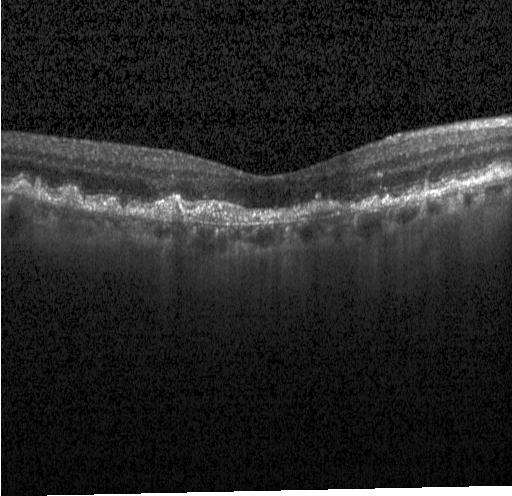
Macular scan · acquired on a Heidelberg Spectralis · retinal OCT cross-section
Dx: CNV.